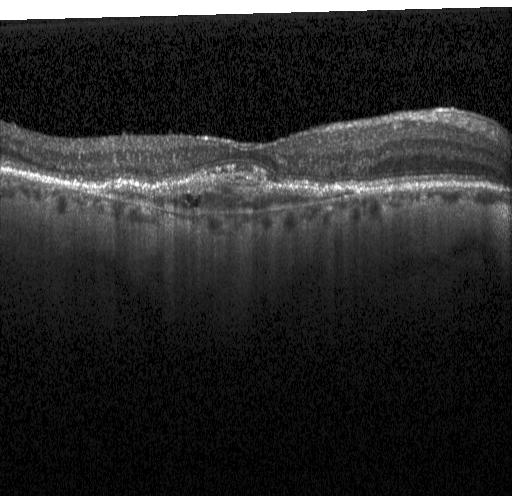
Impression: a choroidal neovascular membrane.